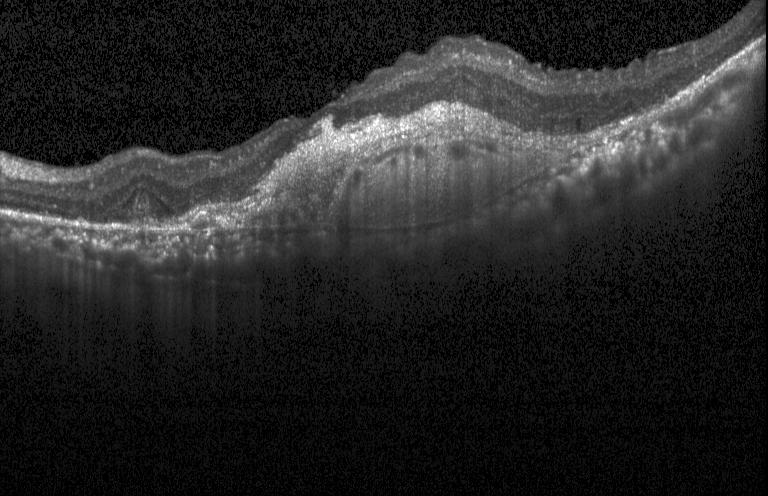
The scan shows choroidal neovascularization.